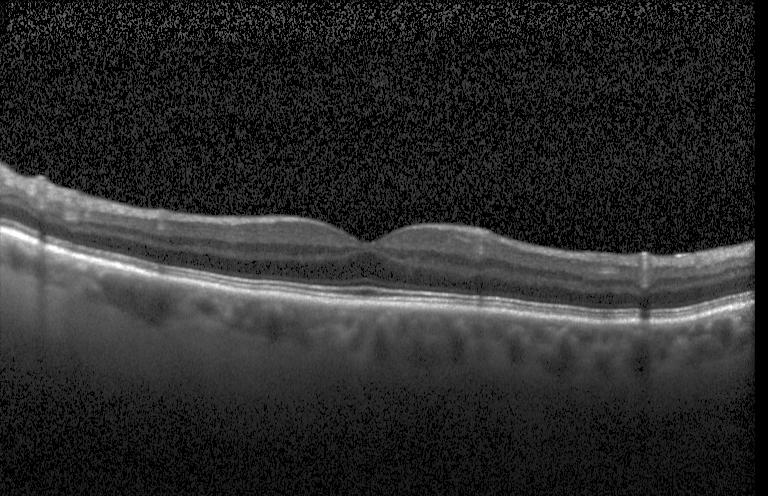 OCT line scan.
Finding: neither choroidal neovascularization, diabetic macular edema, nor drusen.